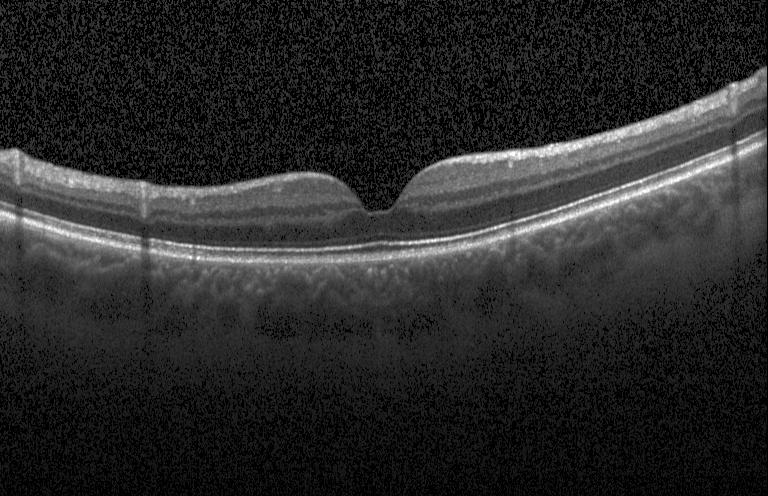
Optical coherence tomography B-scan · Heidelberg Spectralis OCT system. Diagnosis: no evidence of choroidal neovascularization, diabetic macular edema, or drusen.